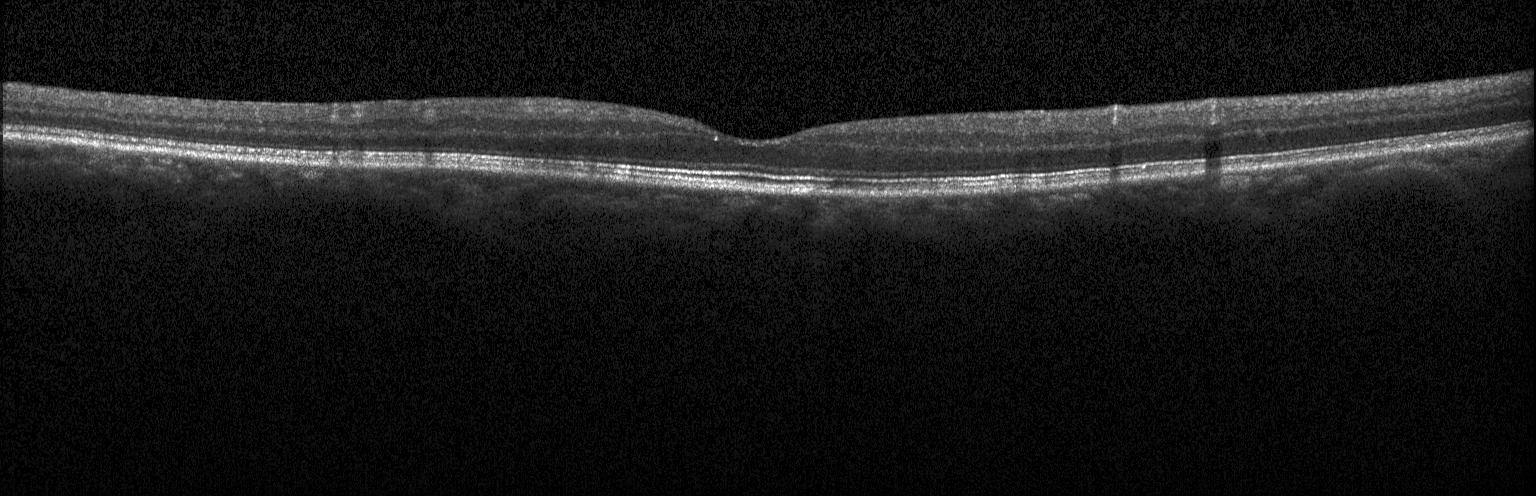
Diagnosis: no choroidal neovascularization, no diabetic macular edema, and no drusen.